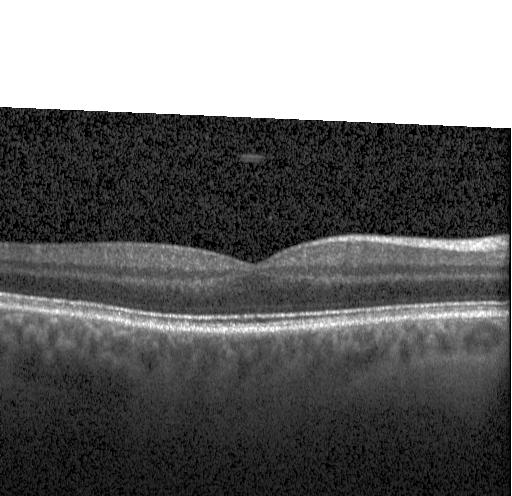
Retinal OCT B-scan.
Finding: no choroidal neovascularization, no diabetic macular edema, and no drusen.